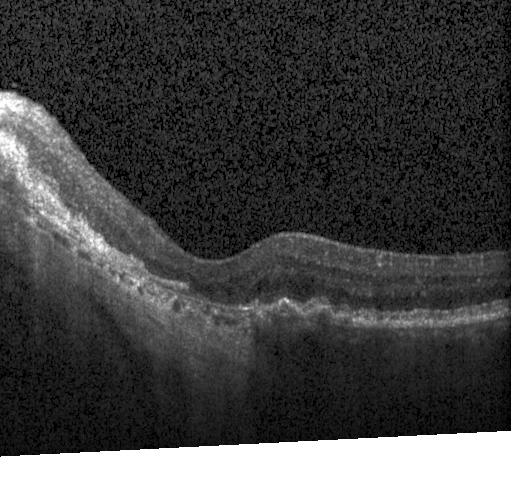

Optical coherence tomography B-scan
The scan shows choroidal neovascularization (CNV).